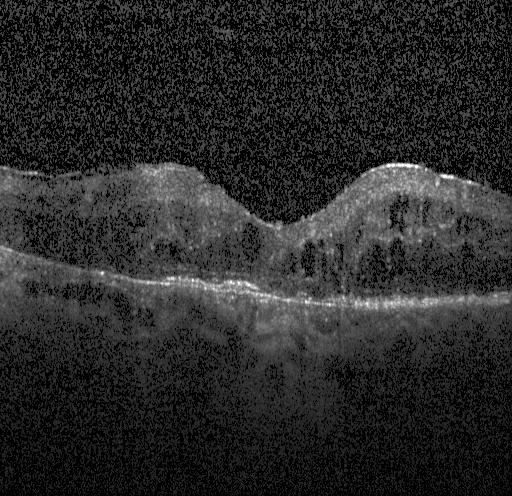

Spectral-domain OCT B-scan: a choroidal neovascular membrane.